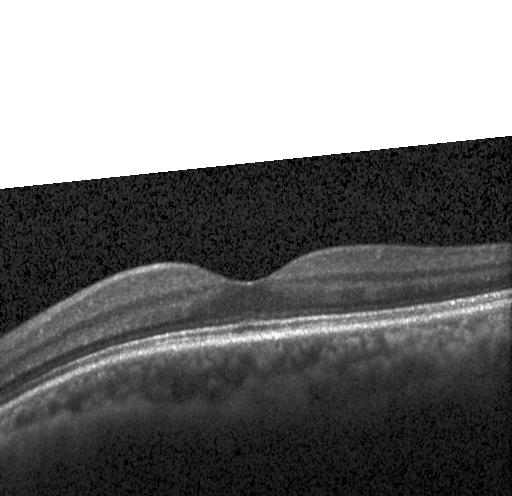

Dx: no evidence of choroidal neovascularization, diabetic macular edema, or drusen.